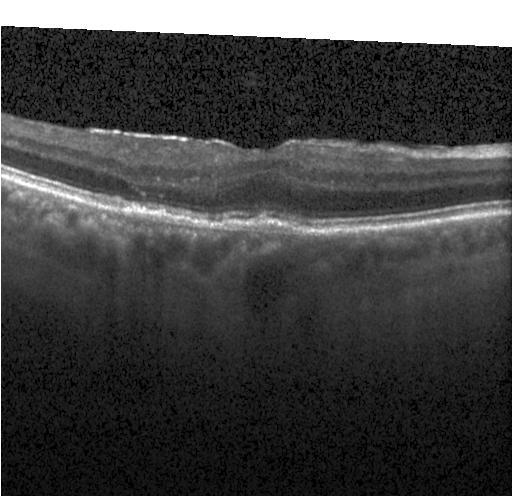 Retinal OCT B-scan · fovea-centered · spectral-domain OCT
This B-scan demonstrates a choroidal neovascular membrane.